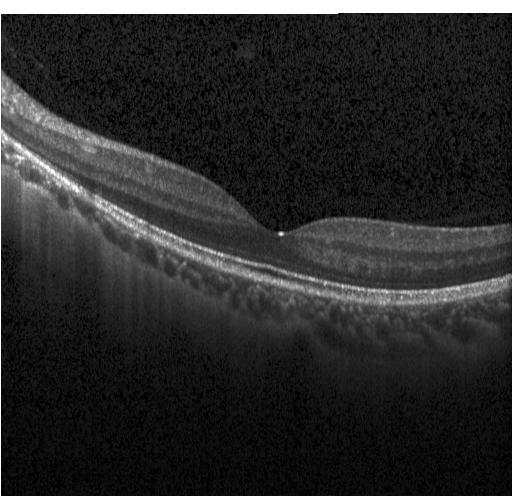
Spectral-domain optical coherence tomography; fovea-centered; Heidelberg Spectralis OCT system; OCT B-scan.
Macular OCT: no CNV, DME, or drusen.